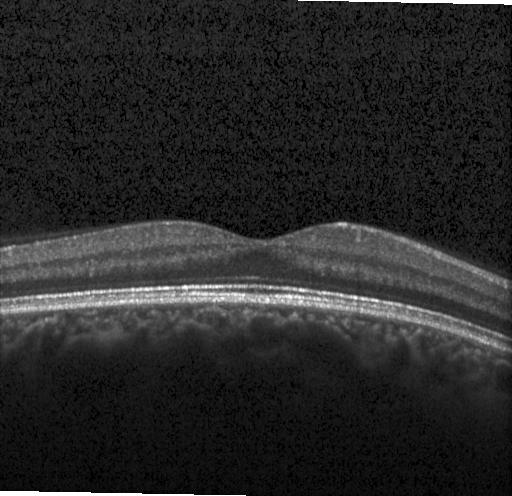
Impression: no choroidal neovascularization, diabetic macular edema, or drusen.